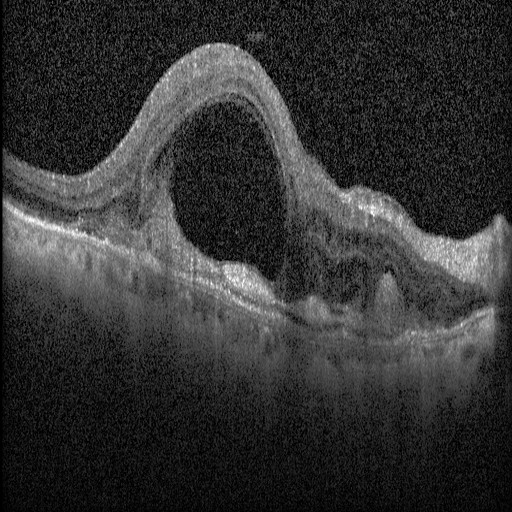
Spectral-domain OCT B-scan: diabetic macular edema (DME).